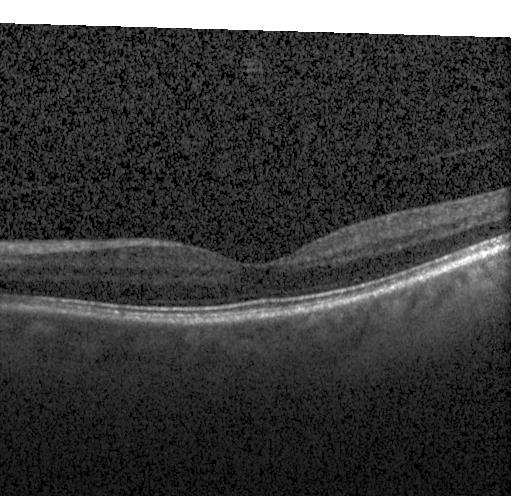

OCT B-scan; spectral-domain optical coherence tomography. Diagnosis: no evidence of choroidal neovascularization, diabetic macular edema, or drusen.